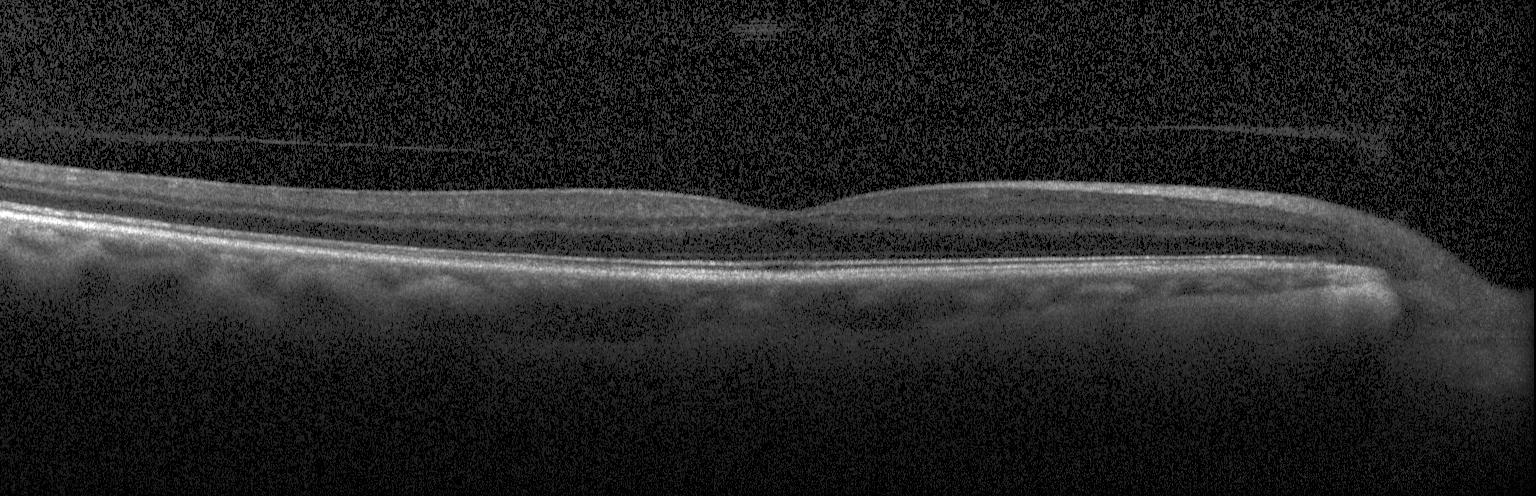
Macular OCT: neither CNV, DME, nor drusen.